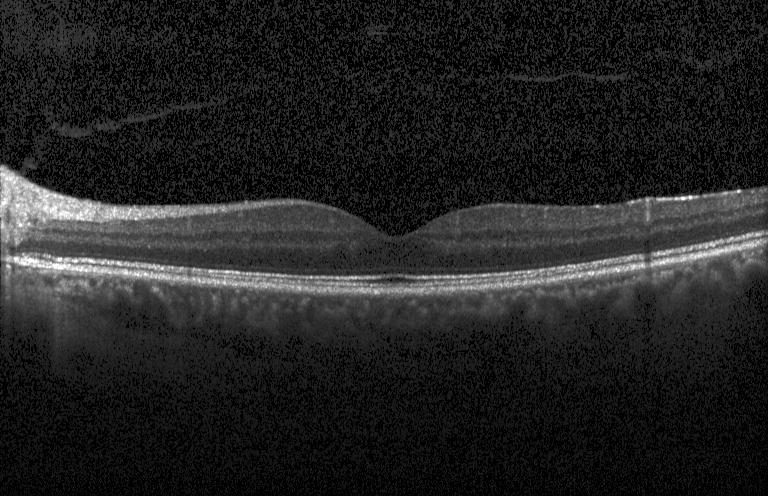
The scan shows no CNV, no DME, and no drusen.